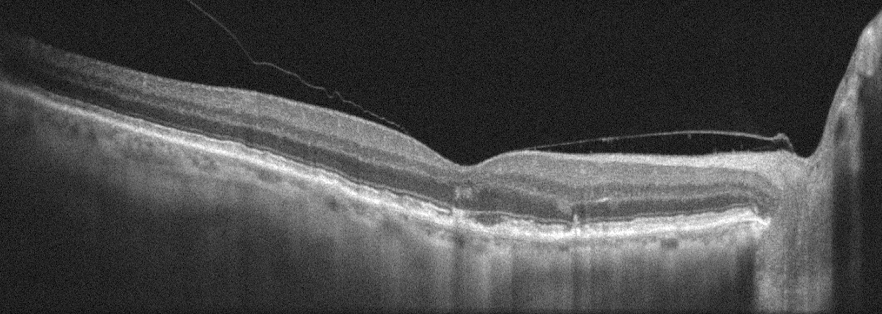 OD; retinal OCT cross-section
This B-scan demonstrates AMD.